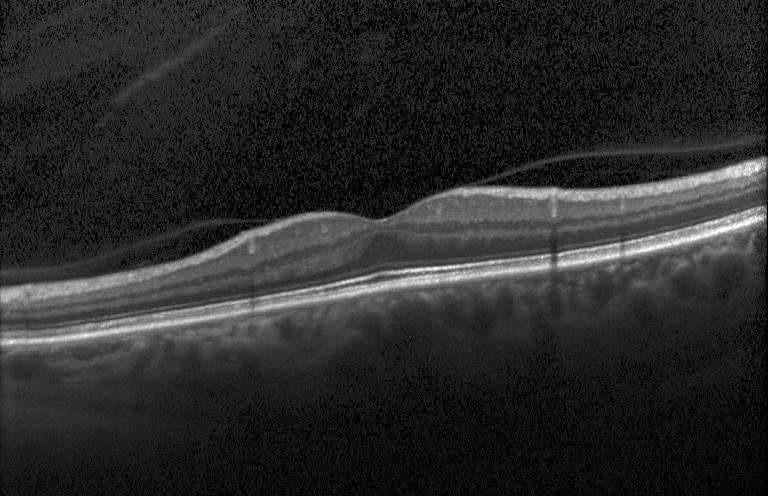

OCT B-scan, SD-OCT, Heidelberg Spectralis OCT system
Dx: neither choroidal neovascularization, diabetic macular edema, nor drusen.